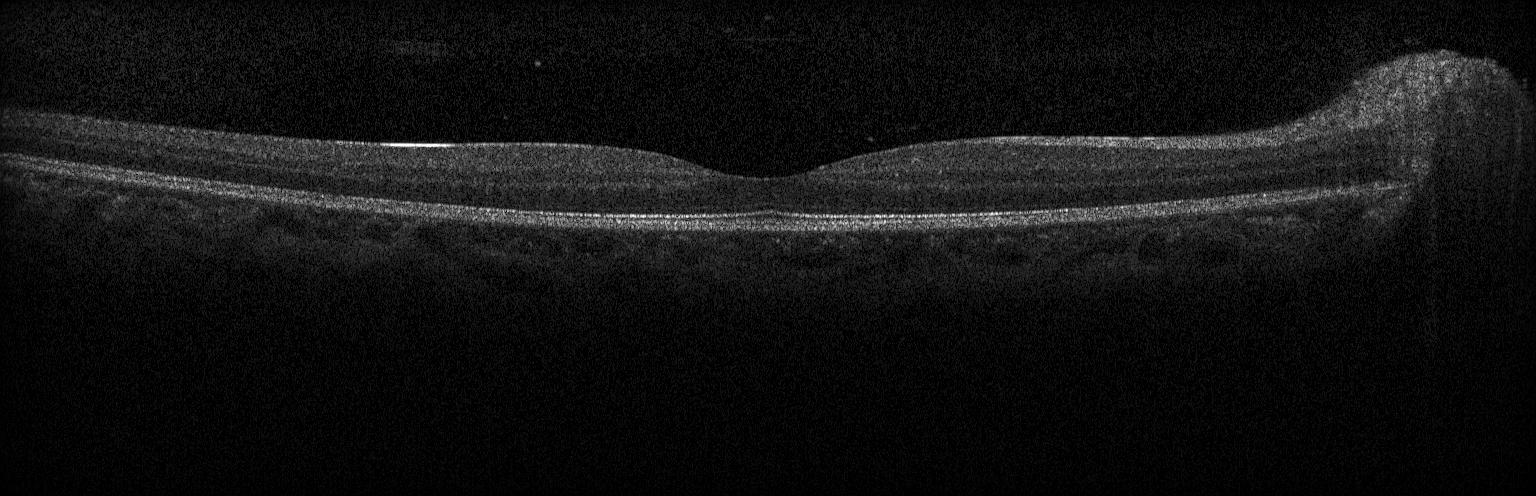

Horizontal scan through the fovea. OCT B-scan. Spectral-domain optical coherence tomography. Instrument: Heidelberg Spectralis. This B-scan demonstrates neither choroidal neovascularization, diabetic macular edema, nor drusen.